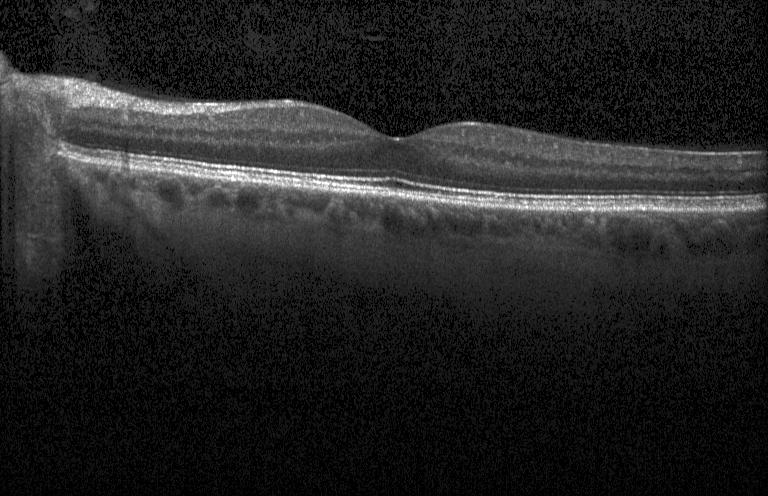
SD-OCT. Optical coherence tomography B-scan. Macular scan
No CNV, DME, or drusen.